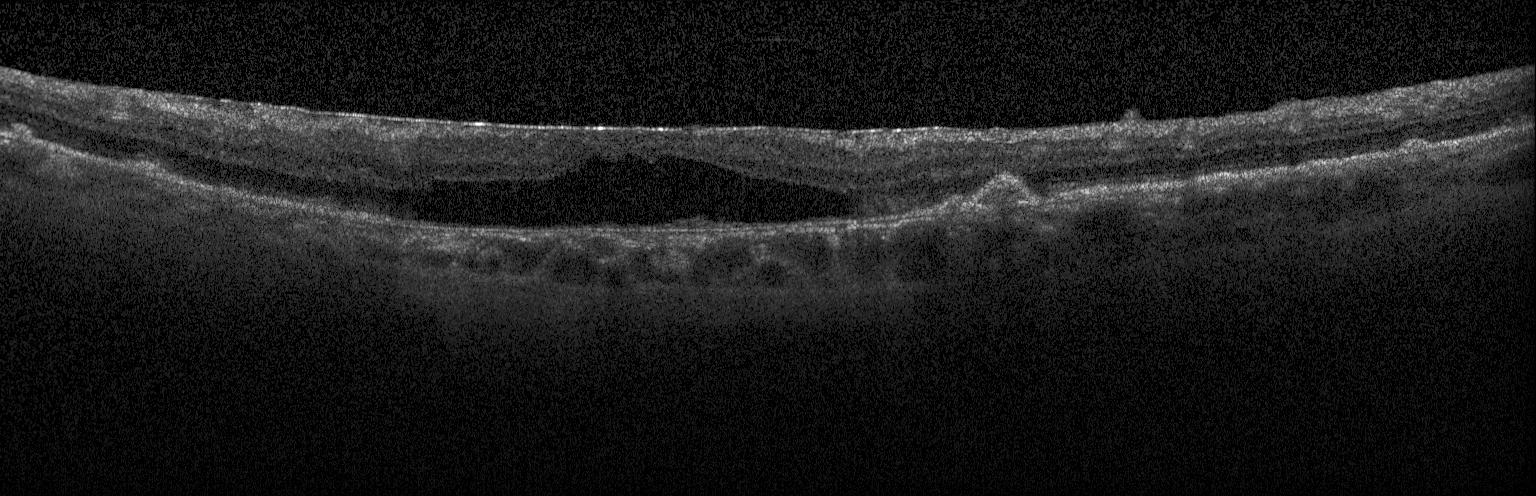
Macular OCT demonstrating a choroidal neovascular membrane.